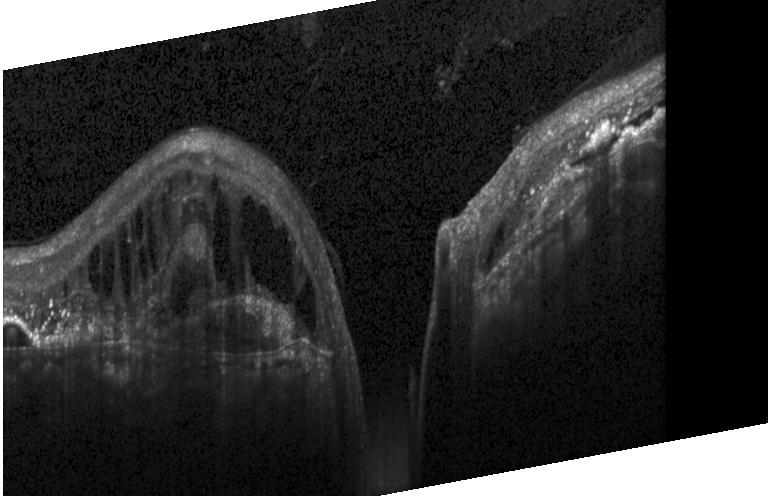
Retinal OCT cross-section. Diagnosis: choroidal neovascularization (CNV).